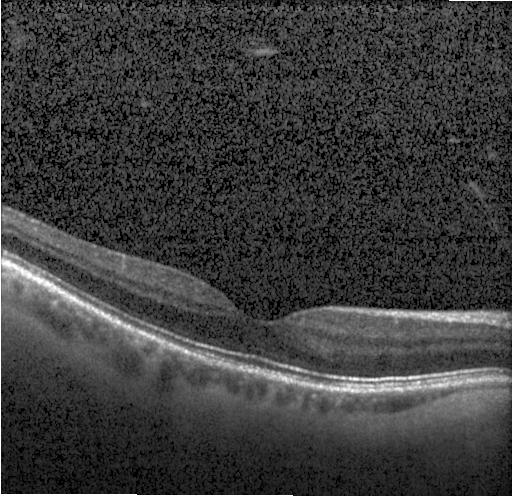 OCT B-scan showing neither CNV, DME, nor drusen.